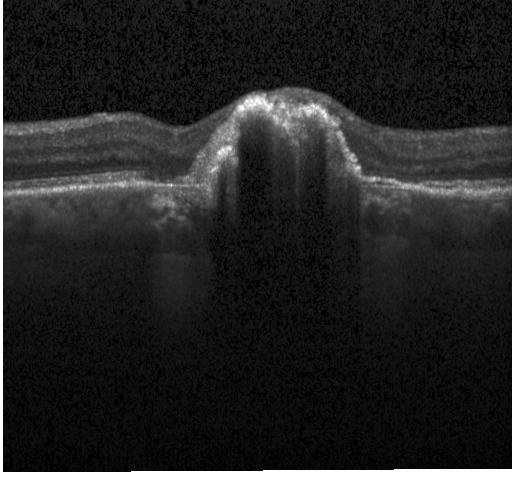
Spectral-domain OCT B-scan: a choroidal neovascular membrane.